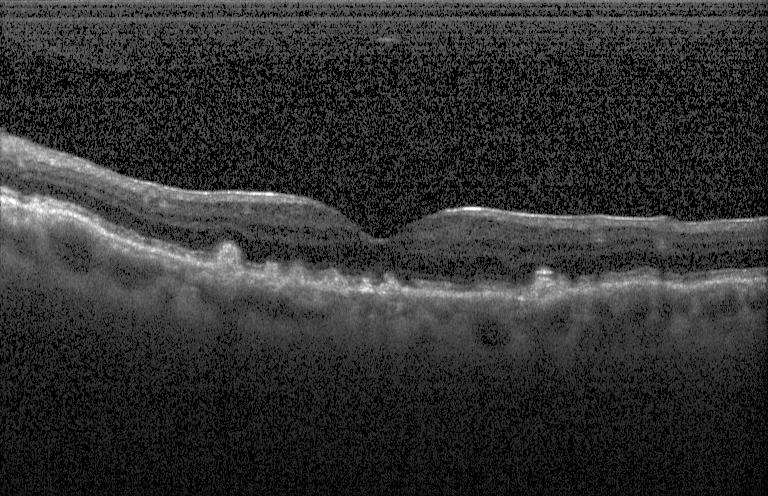
OCT B-scan; instrument: Heidelberg Spectralis. Assessment: sub-RPE drusenoid deposits.